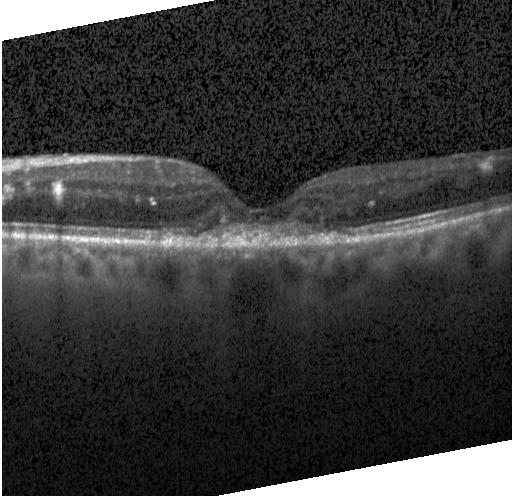 Through the macula · instrument: Heidelberg Spectralis · optical coherence tomography scan
Choroidal neovascularization (CNV).